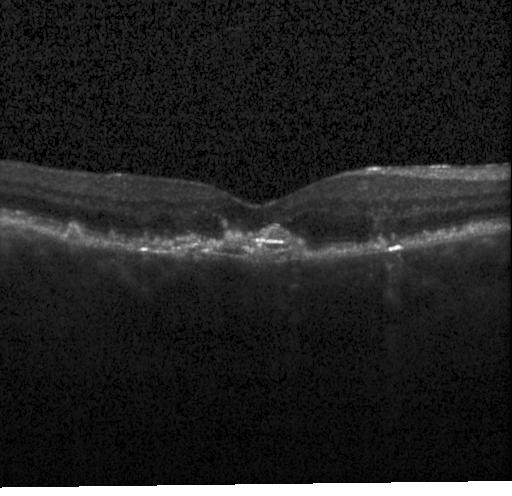 Finding: choroidal neovascularization.